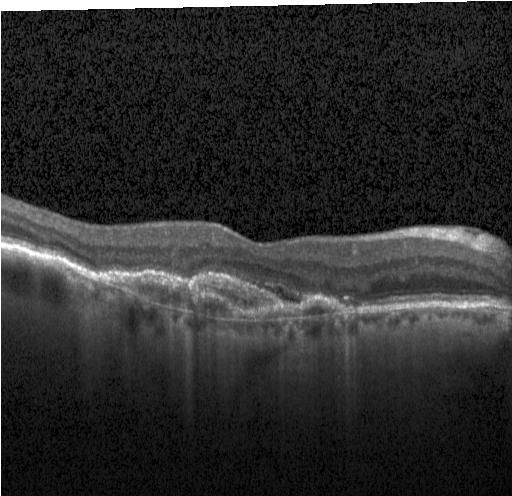 Finding: choroidal neovascularization.